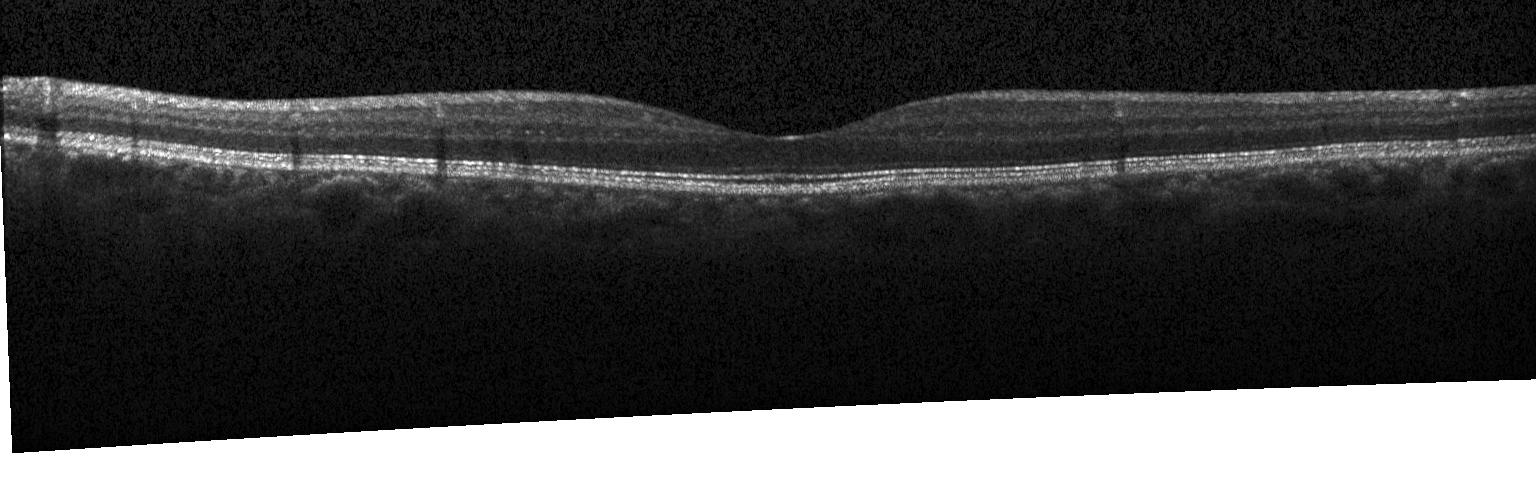
Finding: no evidence of choroidal neovascularization, diabetic macular edema, or drusen.